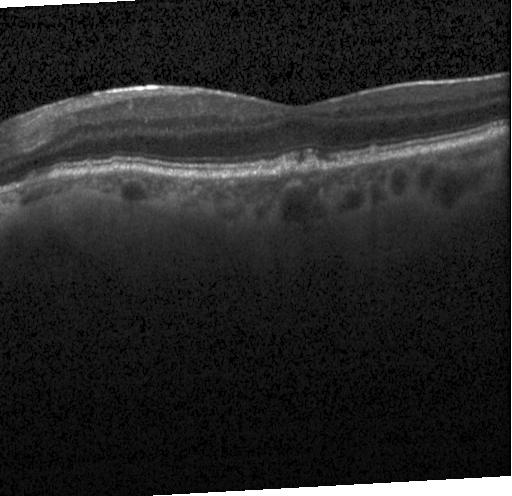 Heidelberg Spectralis OCT system. Fovea-centered. Retinal OCT cross-section. Spectral-domain OCT — Multiple drusen.